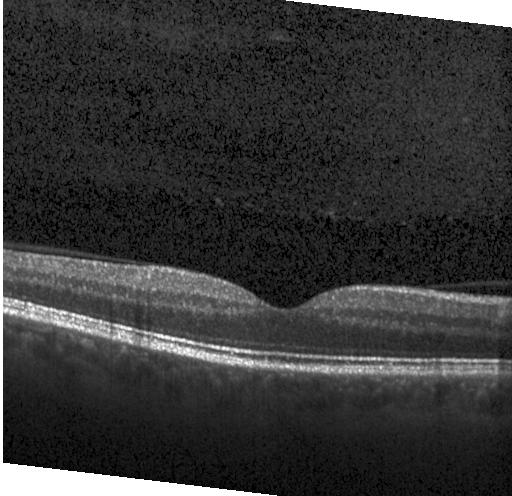

Heidelberg Spectralis; OCT B-scan
The scan shows no CNV, no DME, and no drusen.